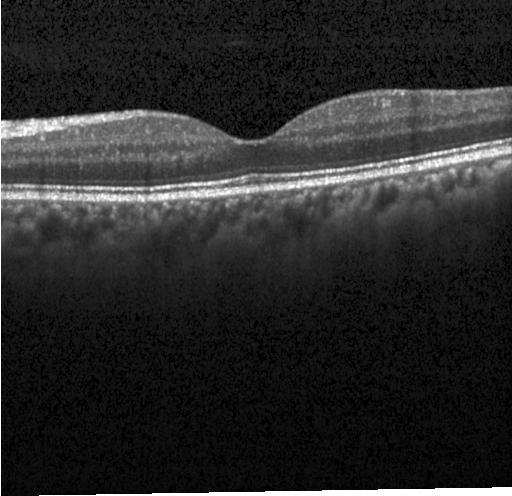 Instrument: Heidelberg Spectralis · macular scan · optical coherence tomography B-scan.
Diagnosis: neither CNV, DME, nor drusen.